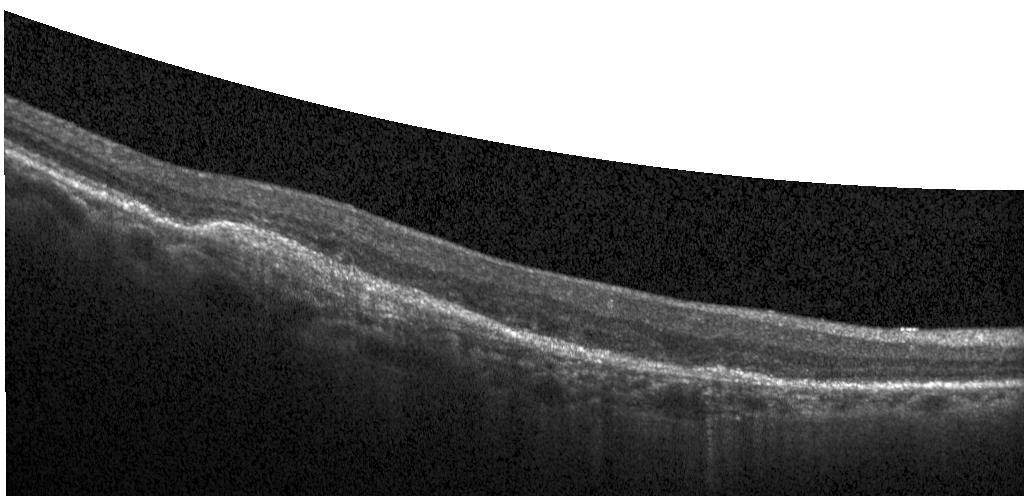

Finding: choroidal neovascularization (CNV).